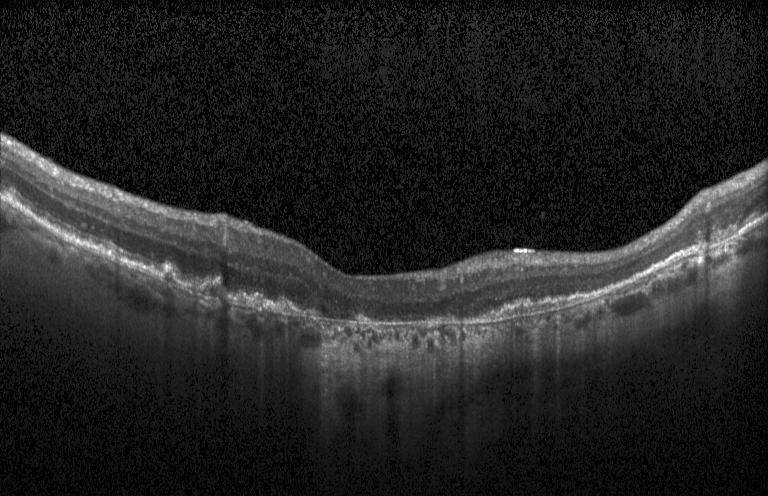 This B-scan demonstrates a choroidal neovascular membrane.